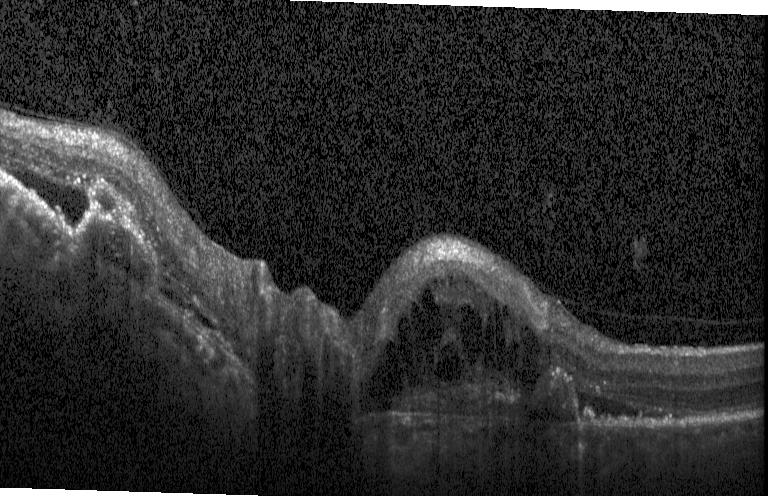 Horizontal scan through the fovea. Optical coherence tomography scan. Spectral-domain OCT. Assessment: a choroidal neovascular membrane.